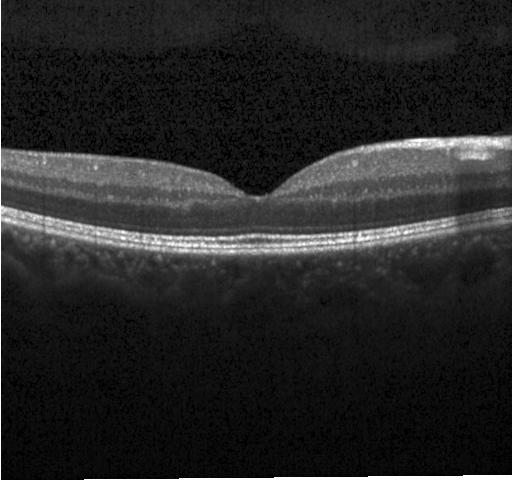
Retinal OCT cross-section.
This B-scan demonstrates no choroidal neovascularization, no diabetic macular edema, and no drusen.